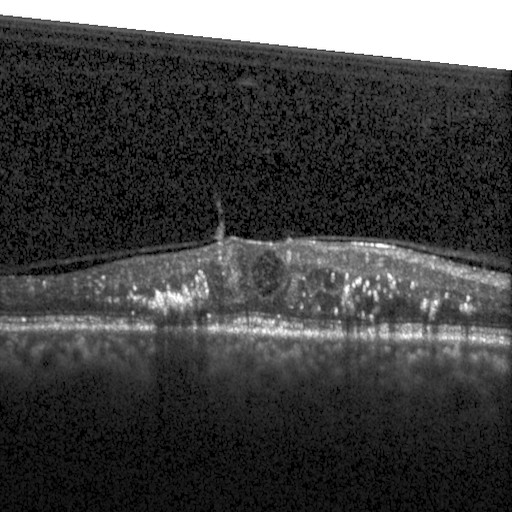

The scan shows diabetic macular edema (DME).